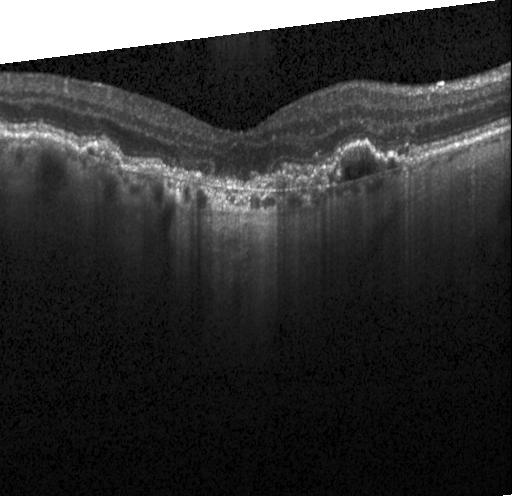

Acquired on a Heidelberg Spectralis, OCT line scan
Choroidal neovascularization.